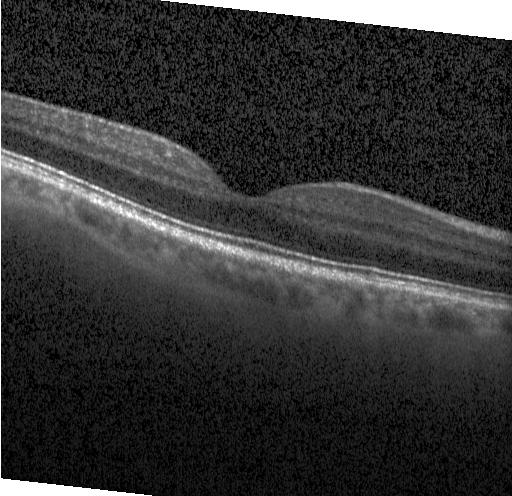 Fovea-centered, optical coherence tomography scan, SD-OCT
Impression: no CNV, no DME, and no drusen.